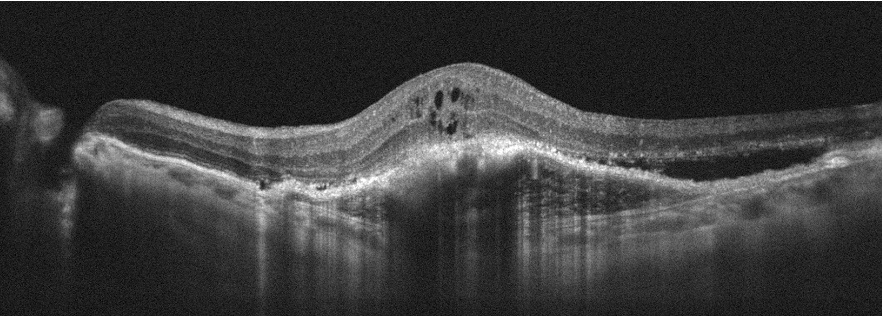 Impression: age-related macular degeneration (AMD).